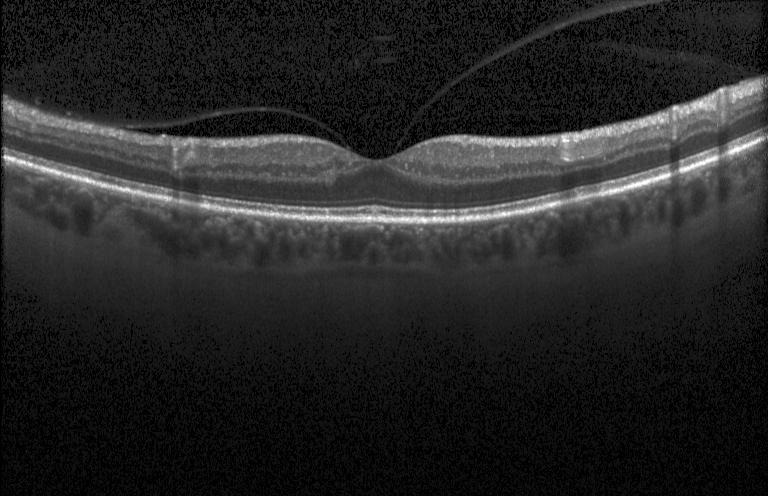

Neither choroidal neovascularization, diabetic macular edema, nor drusen.